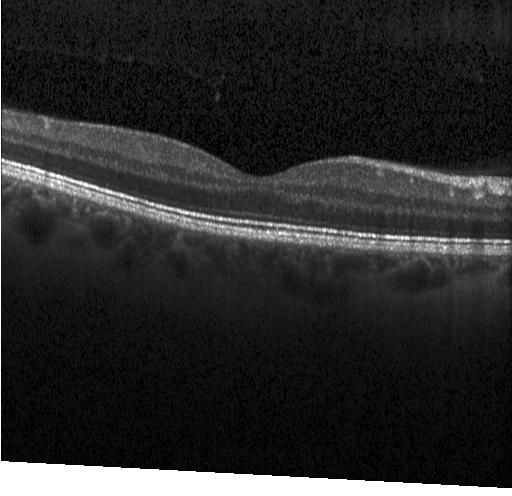
Macular OCT: no choroidal neovascularization, no diabetic macular edema, and no drusen.